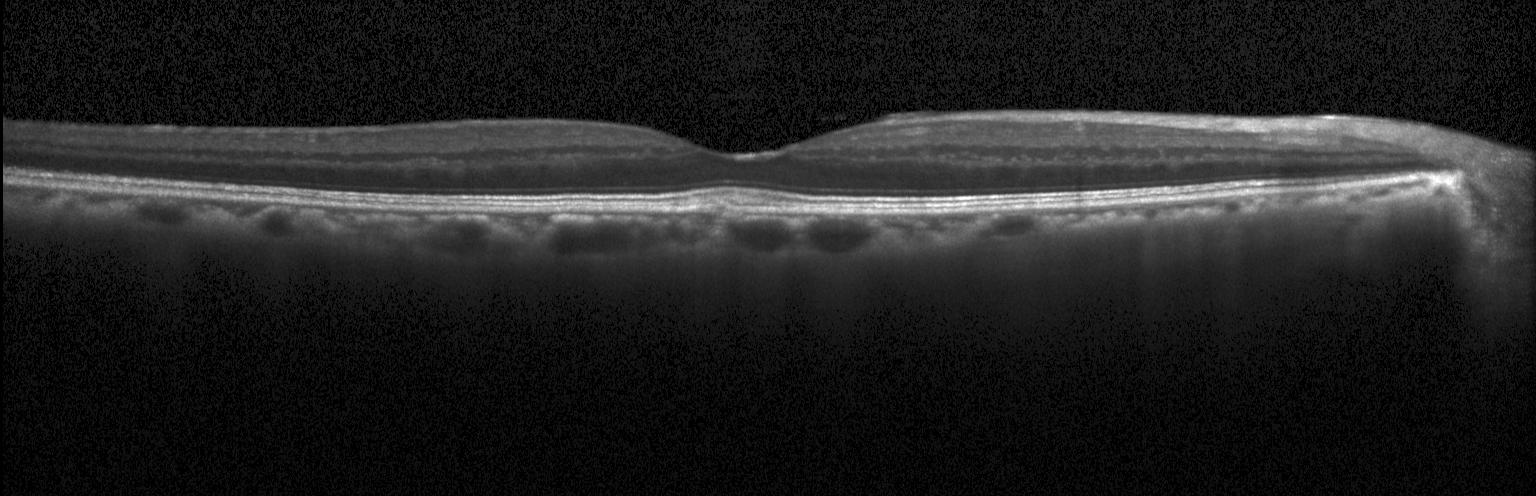
SD-OCT; optical coherence tomography scan; fovea-centered
Finding: neither CNV, DME, nor drusen.